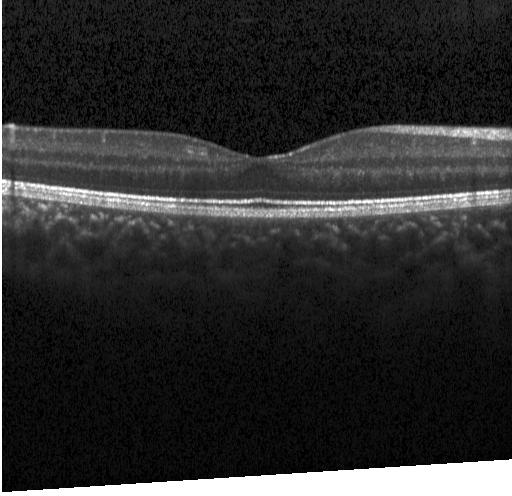 Dx: no CNV, no DME, and no drusen.